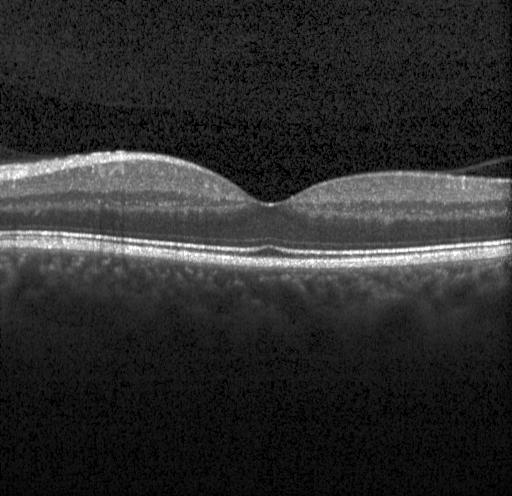

OCT line scan — Impression: neither choroidal neovascularization, diabetic macular edema, nor drusen.